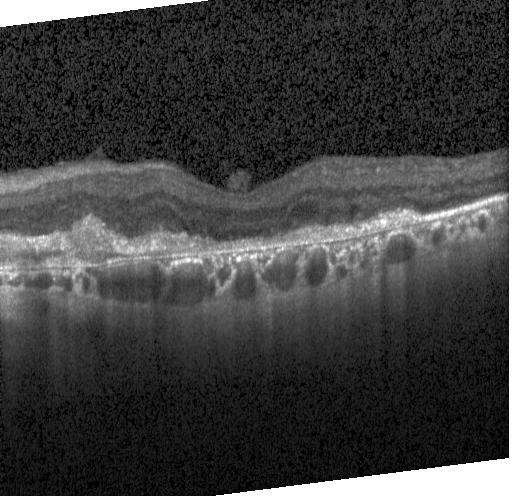 Diagnosis: choroidal neovascularization (CNV).